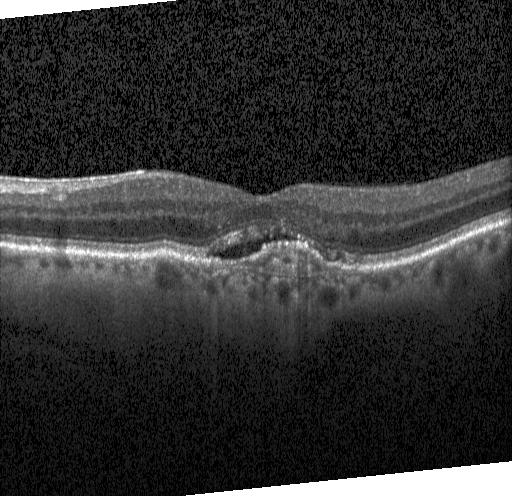

Horizontal scan through the fovea; instrument: Heidelberg Spectralis; optical coherence tomography B-scan — Macular OCT: CNV.